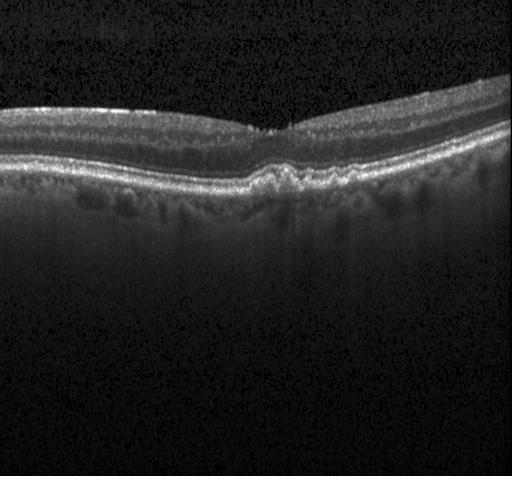

Macular scan; optical coherence tomography B-scan.
Impression: multiple drusen.